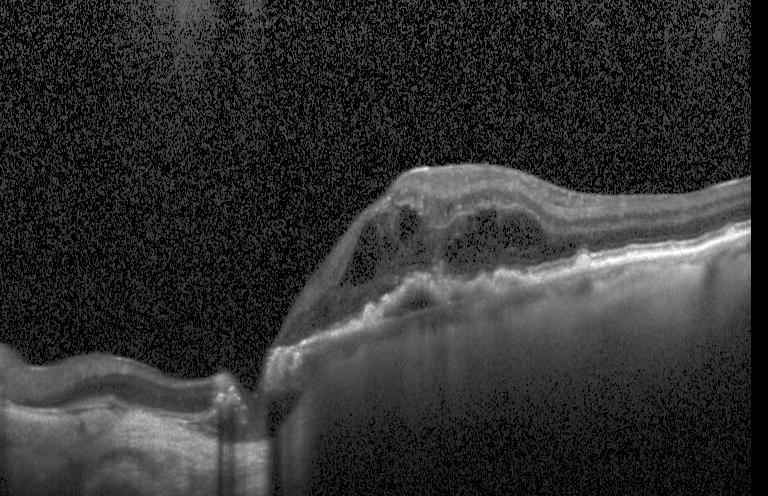

Finding: a choroidal neovascular membrane.